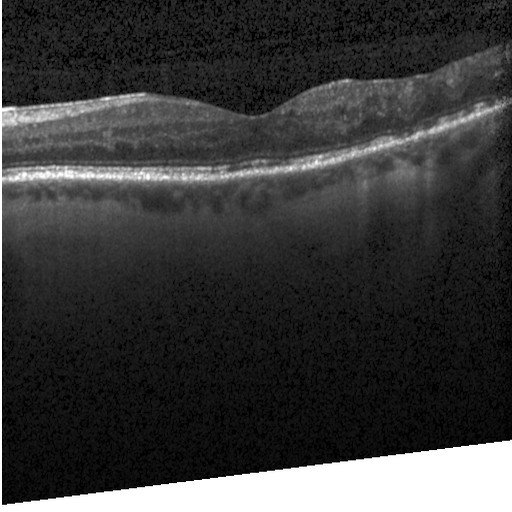

Impression: diabetic macular edema (DME).